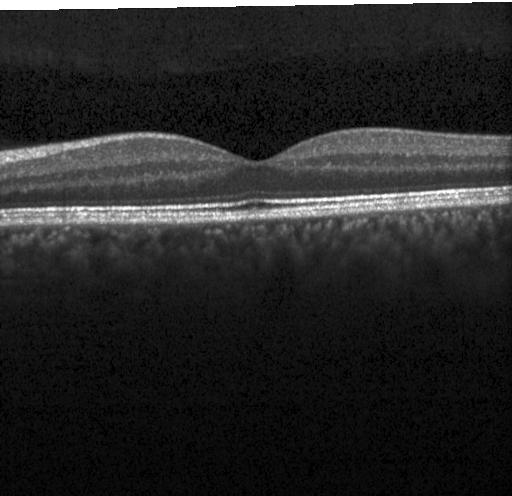
Spectral-domain OCT. Heidelberg Spectralis. Retinal OCT B-scan
No choroidal neovascularization, diabetic macular edema, or drusen.